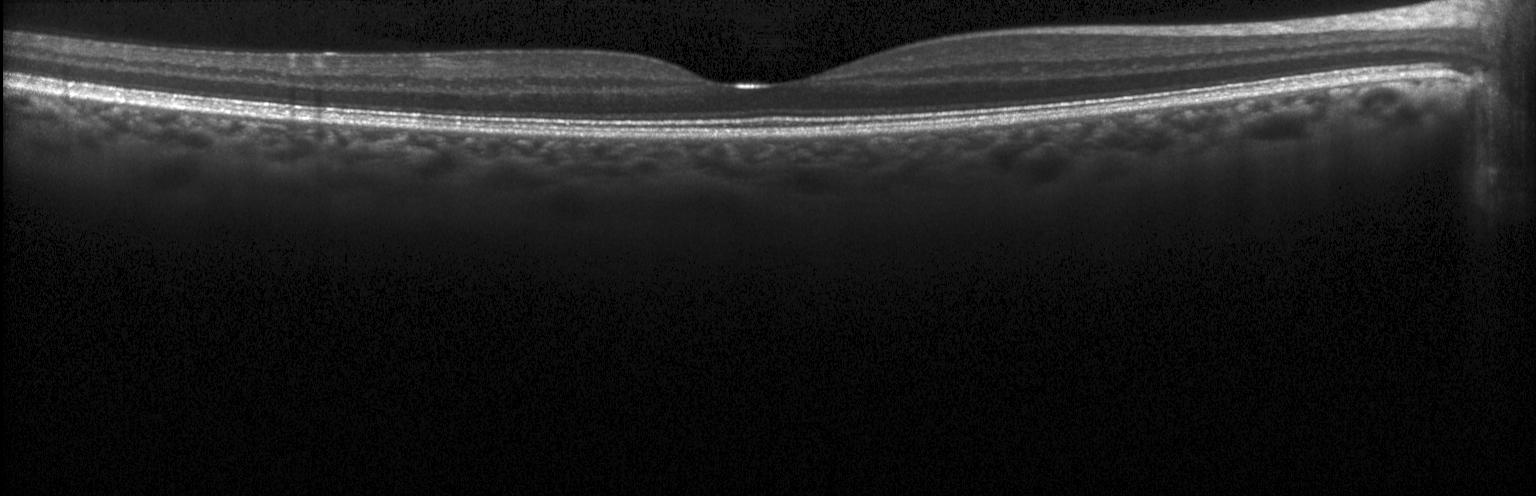 Impression: no evidence of choroidal neovascularization, diabetic macular edema, or drusen.